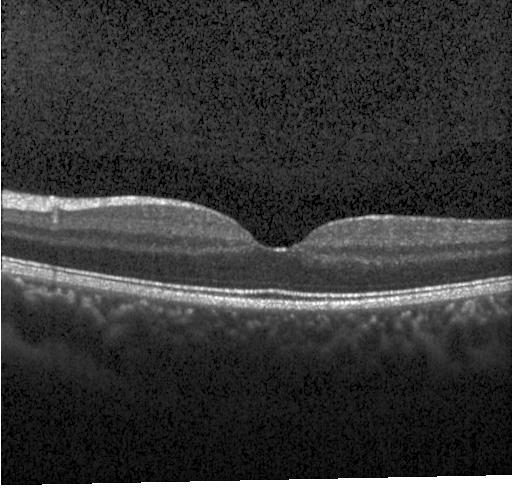
Horizontal scan through the fovea; Heidelberg Spectralis; OCT B-scan — Finding: no evidence of choroidal neovascularization, diabetic macular edema, or drusen.